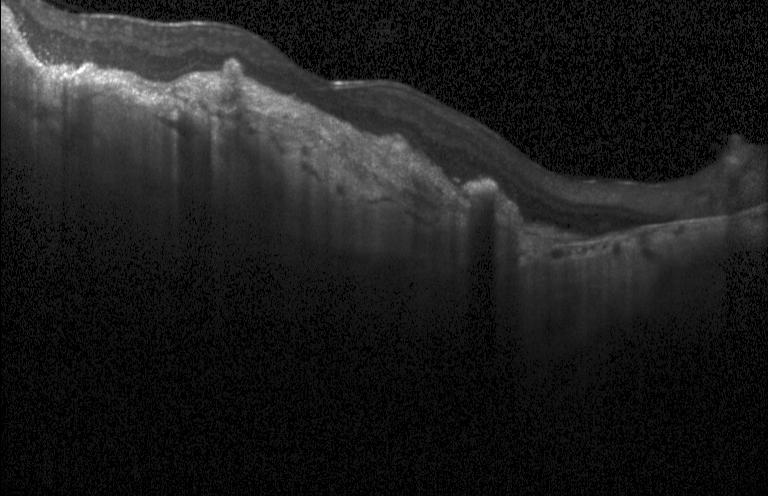 Heidelberg Spectralis OCT system; retinal OCT cross-section; spectral-domain optical coherence tomography; centered on the fovea — Diagnosis: a choroidal neovascular membrane.